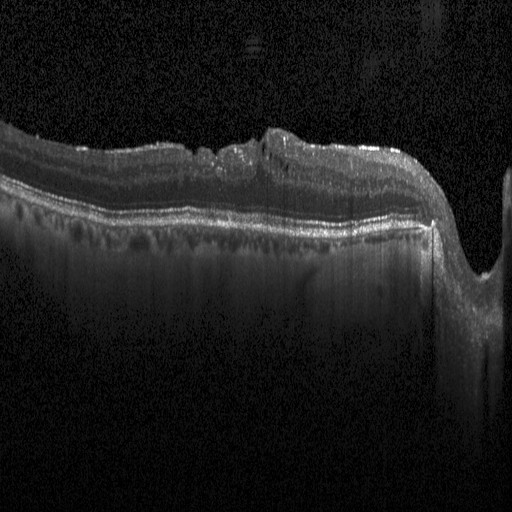 Optical coherence tomography scan; spectral-domain OCT — Macular OCT: diabetic macular edema.